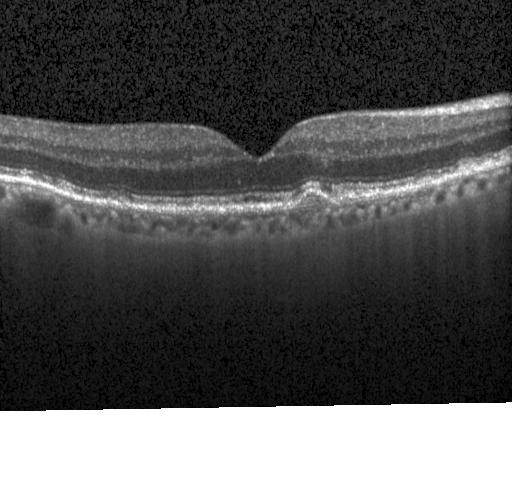
Diagnosis: multiple drusen.